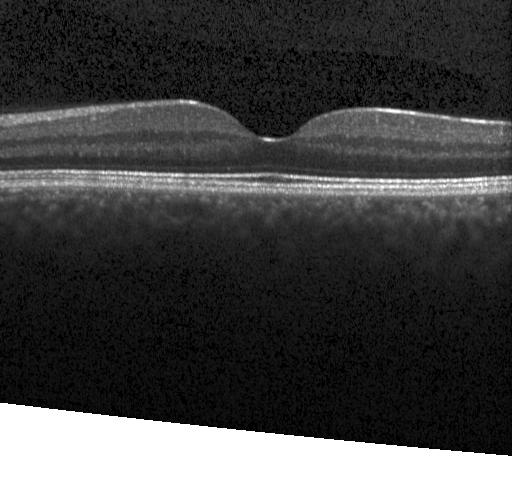
Retinal OCT B-scan; spectral-domain optical coherence tomography; horizontal scan through the fovea
No evidence of choroidal neovascularization, diabetic macular edema, or drusen.